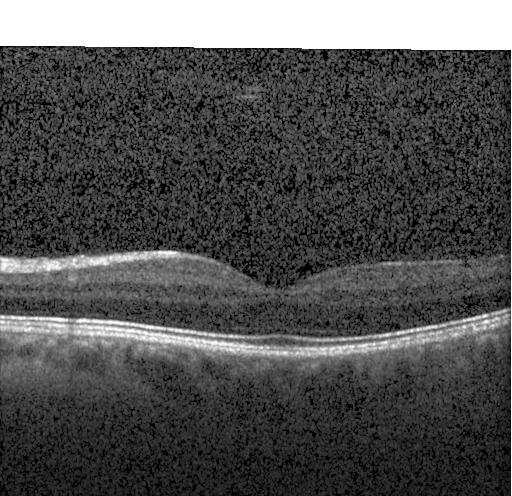

Spectral-domain OCT B-scan: neither CNV, DME, nor drusen.